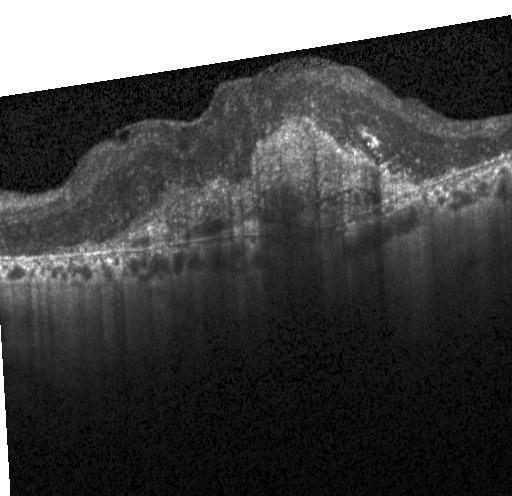 Heidelberg Spectralis OCT system; spectral-domain OCT; horizontal scan through the fovea; retinal OCT B-scan.
Impression: choroidal neovascularization (CNV).